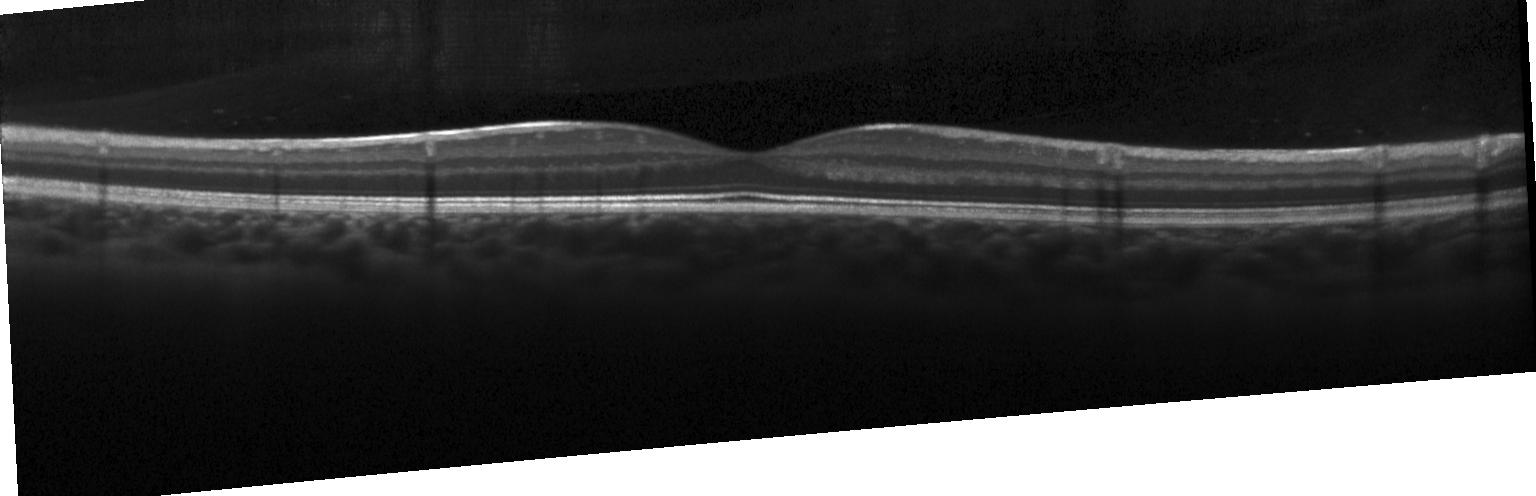
Optical coherence tomography scan
The scan shows no choroidal neovascularization, no diabetic macular edema, and no drusen.